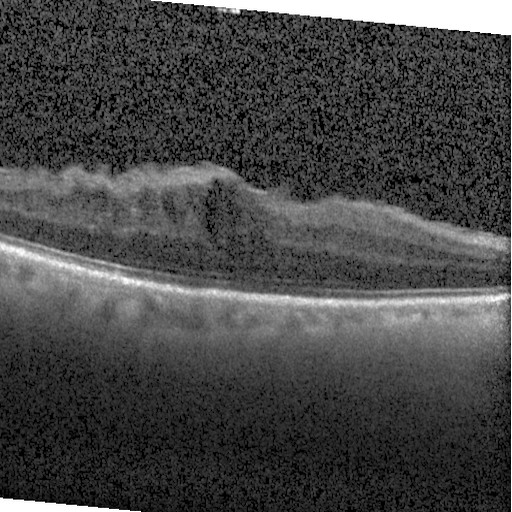
OCT scan showing diabetic macular edema.